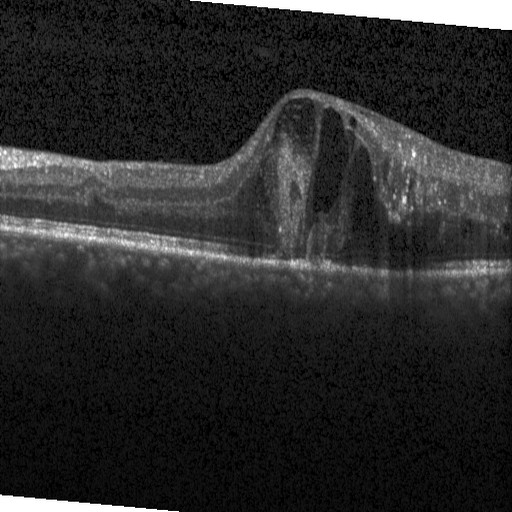 Instrument: Heidelberg Spectralis, retinal OCT B-scan, SD-OCT, macular scan.
This B-scan demonstrates diabetic macular edema.